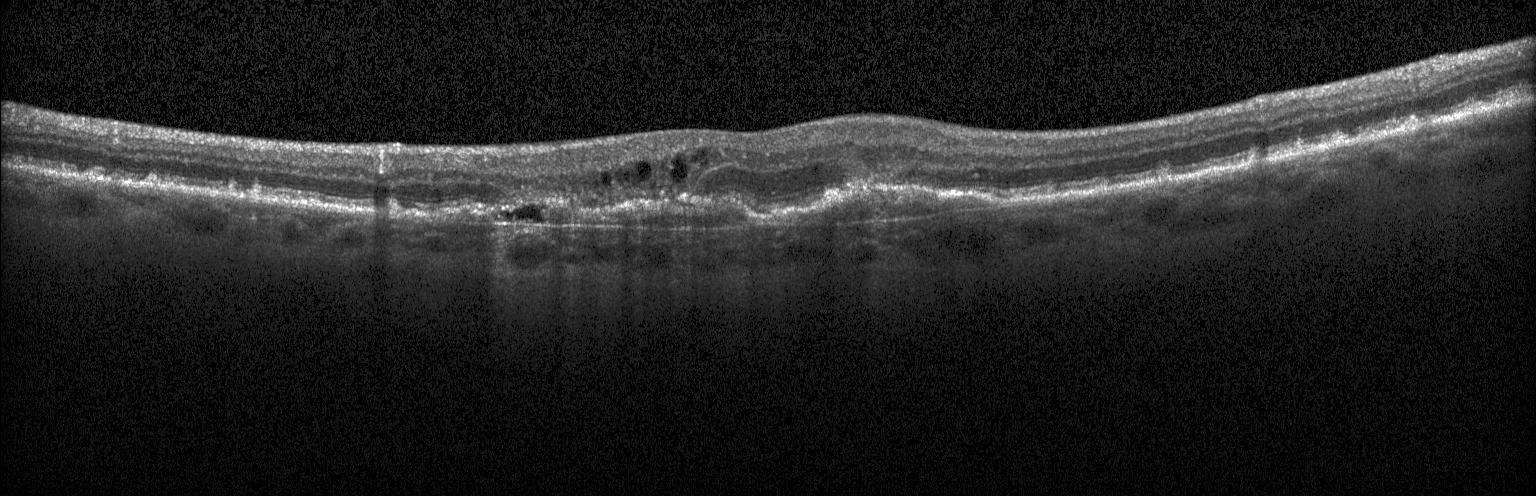

Retinal OCT B-scan — A choroidal neovascular membrane.